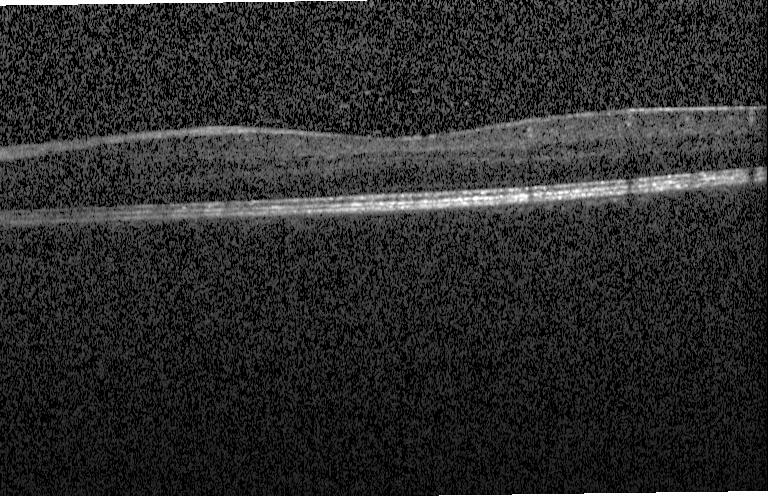 Instrument: Heidelberg Spectralis · optical coherence tomography scan.
No evidence of CNV, DME, or drusen.